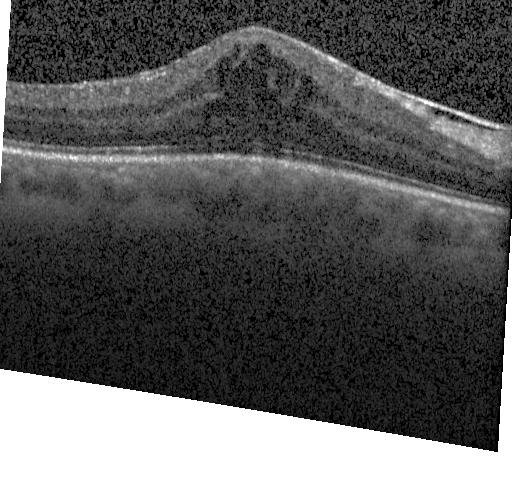 Spectral-domain OCT, fovea-centered, optical coherence tomography scan
The scan shows diabetic macular edema.